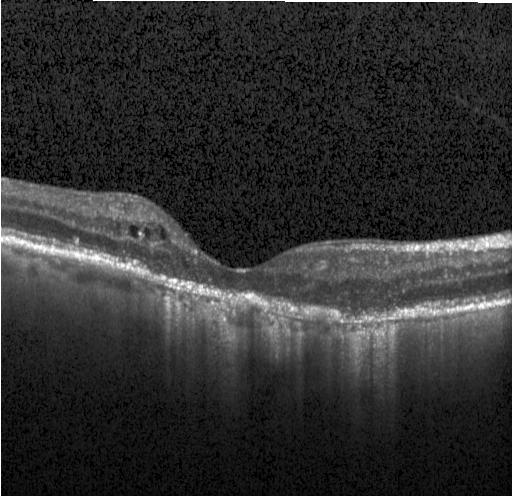 Spectral-domain OCT B-scan: CNV.